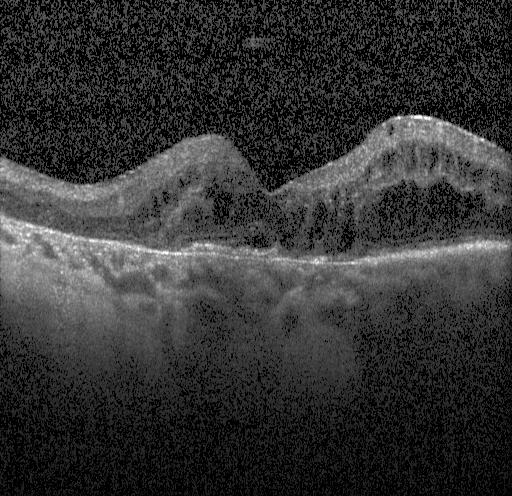 Heidelberg Spectralis OCT system · OCT B-scan · spectral-domain OCT · horizontal scan through the fovea.
Impression: CNV.